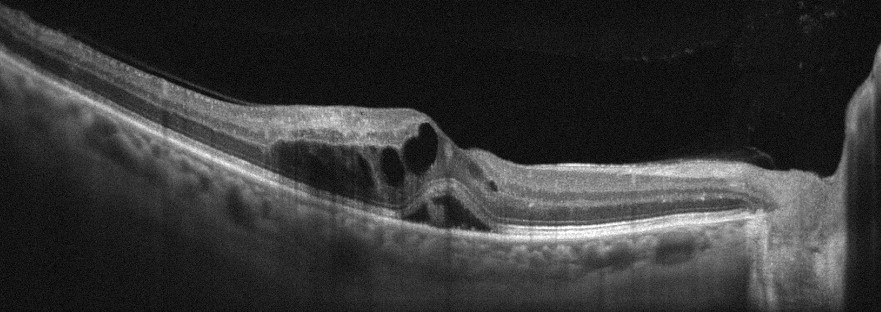
Spectral-domain OCT B-scan: RVO.